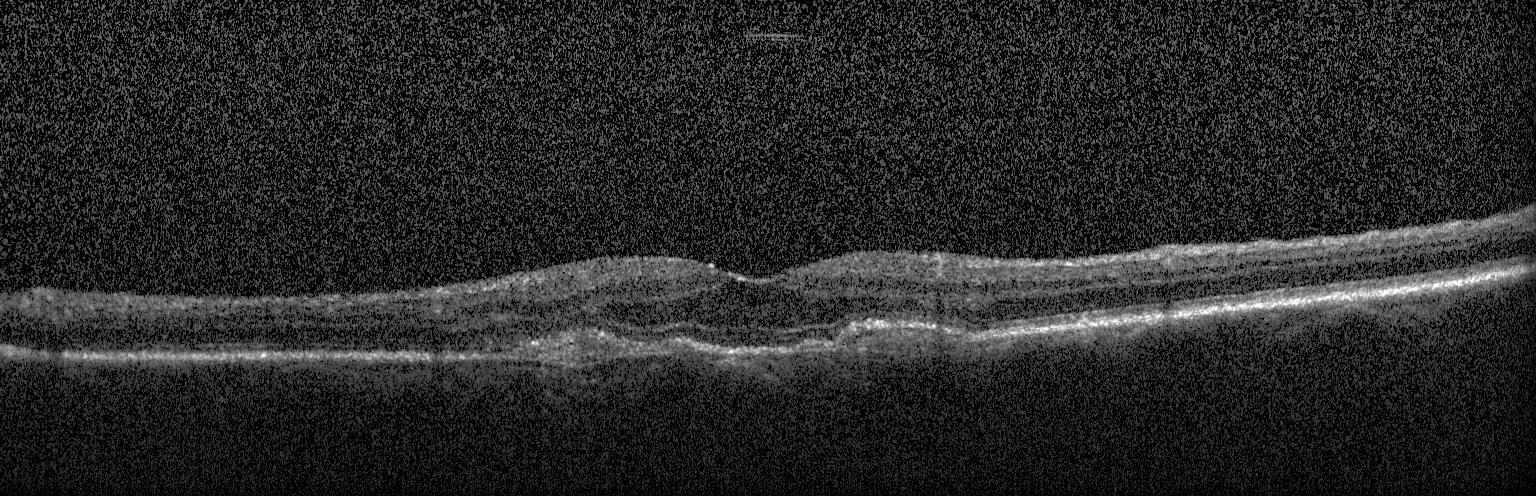 Optical coherence tomography B-scan, spectral-domain OCT.
Finding: a choroidal neovascular membrane.